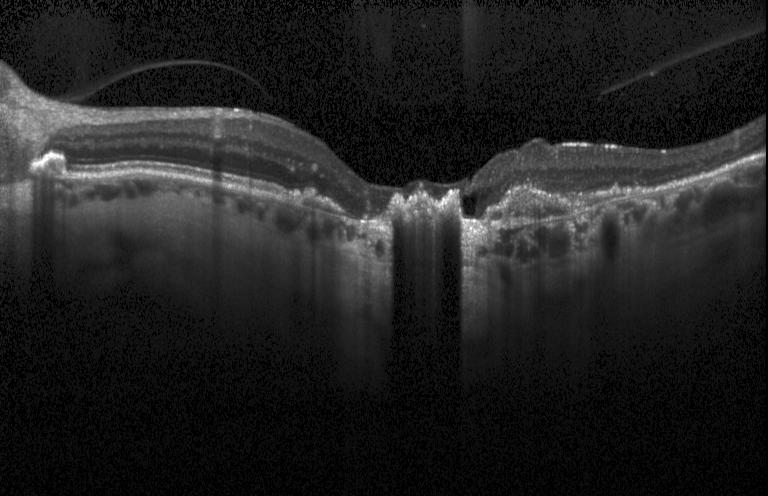 Heidelberg Spectralis; spectral-domain OCT; macular scan; OCT B-scan
Impression: a choroidal neovascular membrane.